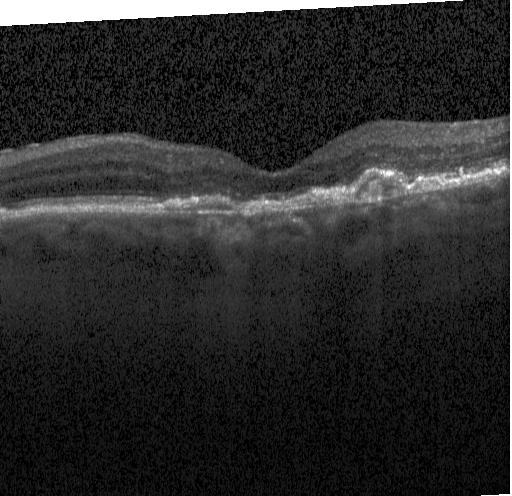 This B-scan demonstrates choroidal neovascularization (CNV).